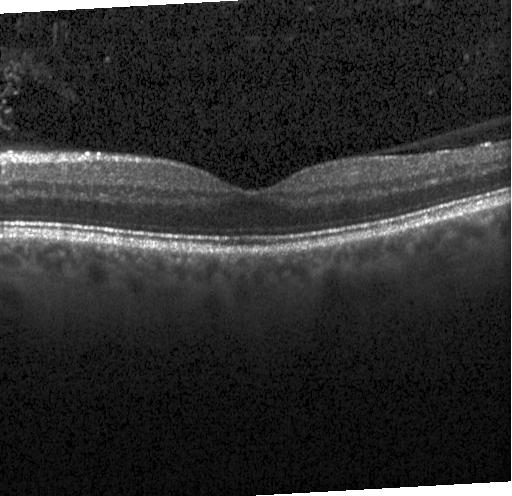
OCT B-scan.
Macular OCT: no evidence of choroidal neovascularization, diabetic macular edema, or drusen.